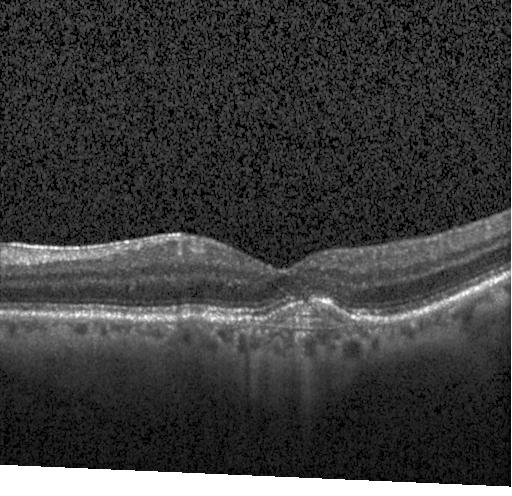
Finding: a choroidal neovascular membrane.